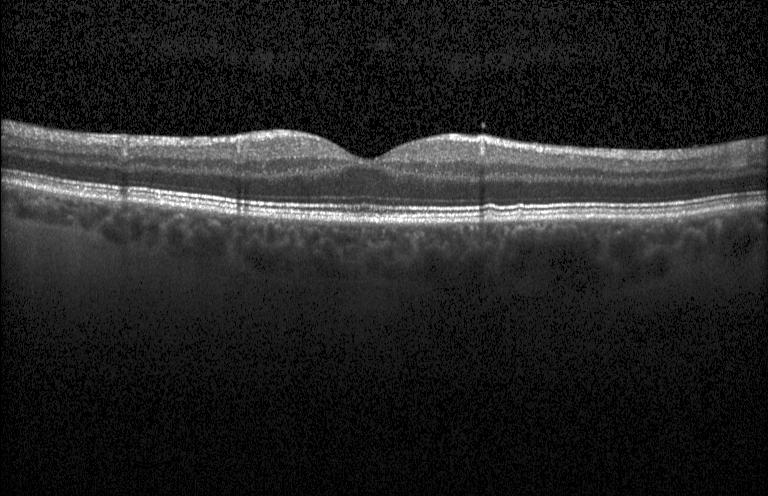

Retinal OCT cross-section — No choroidal neovascularization, diabetic macular edema, or drusen.